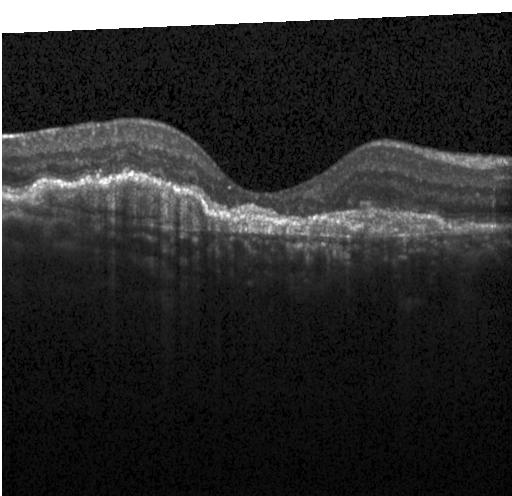
Impression: a choroidal neovascular membrane.